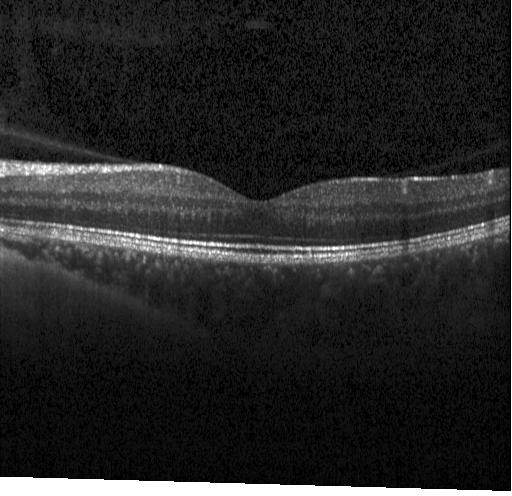
Retinal OCT cross-section
Finding: neither CNV, DME, nor drusen.